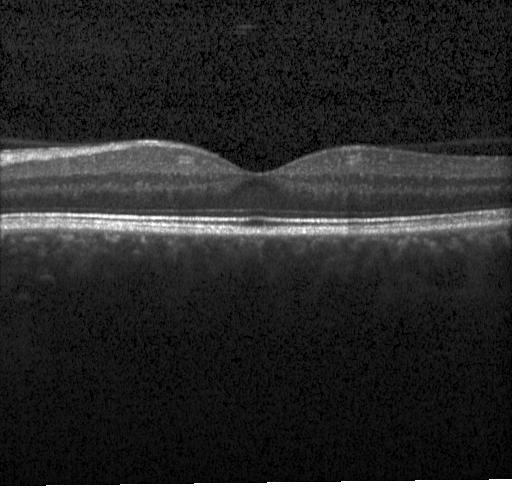 Horizontal scan through the fovea; Heidelberg Spectralis OCT system; optical coherence tomography scan; spectral-domain OCT — Finding: no CNV, DME, or drusen.